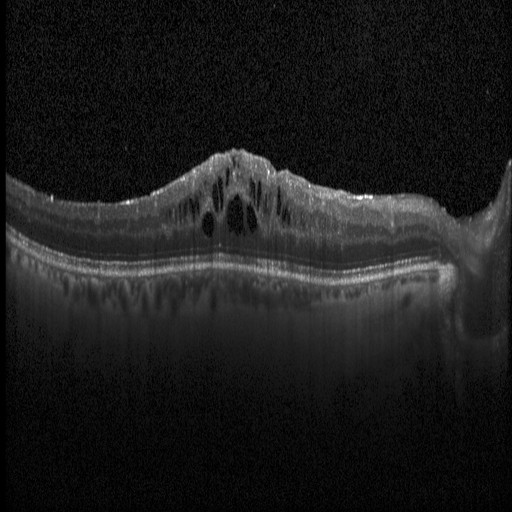
SD-OCT. Optical coherence tomography B-scan
Impression: diabetic macular edema (DME).